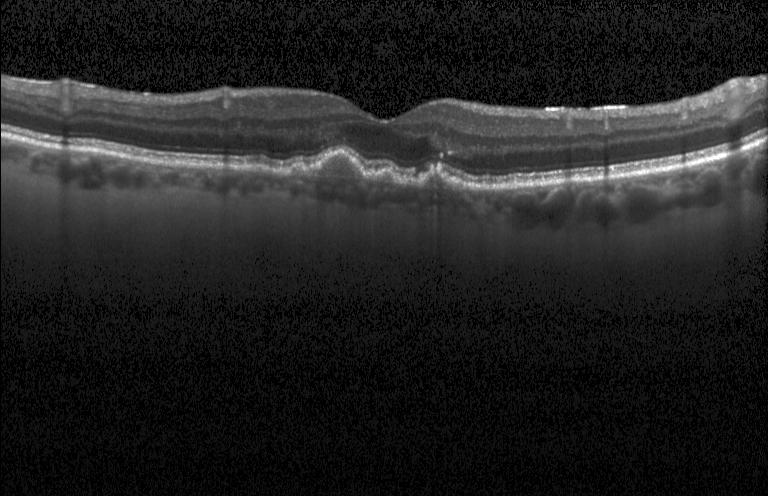 OCT line scan. Instrument: Heidelberg Spectralis. Spectral-domain OCT. Horizontal scan through the fovea. Impression: drusen.